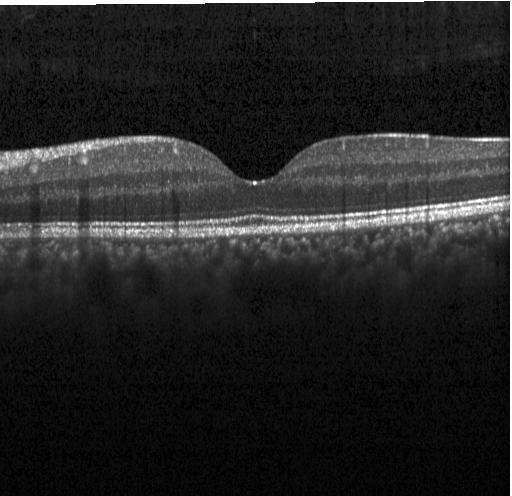 Heidelberg Spectralis · OCT line scan. Diagnosis: no evidence of choroidal neovascularization, diabetic macular edema, or drusen.